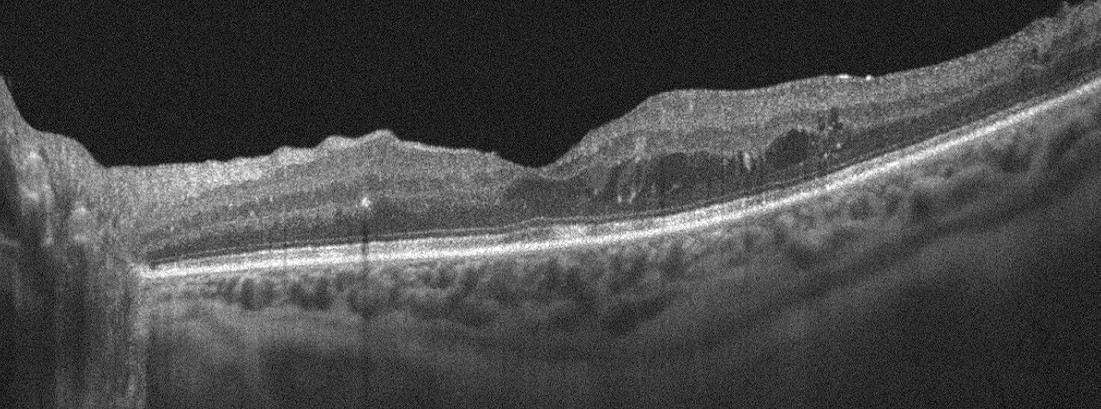

Acquired on an Optovue Avanti RTVue XR · OCT line scan · macular scan. Dx: diabetic macular edema.